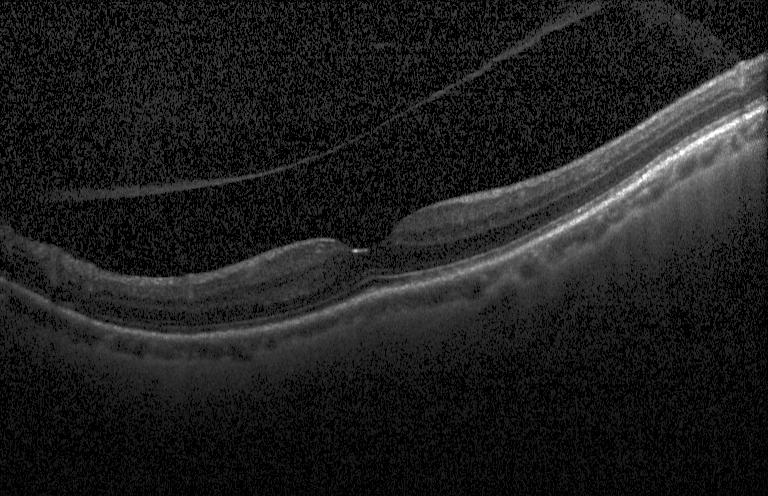
Centered on the fovea; spectral-domain optical coherence tomography; optical coherence tomography scan
Dx: no choroidal neovascularization, diabetic macular edema, or drusen.